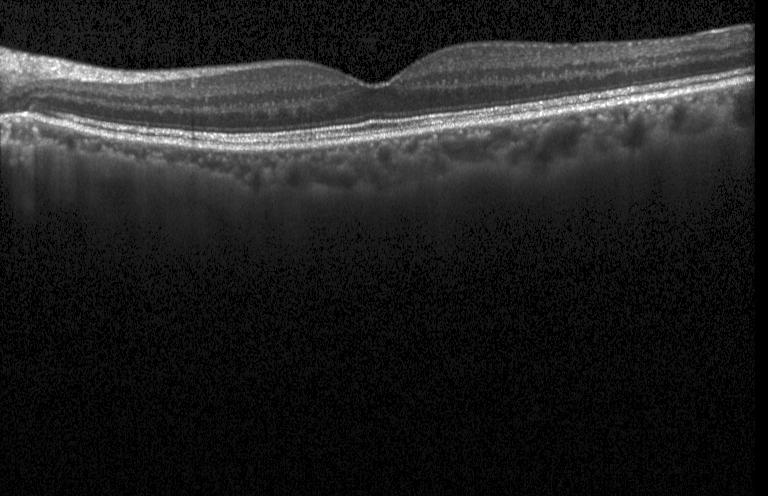
Instrument: Heidelberg Spectralis. Optical coherence tomography scan
Impression: no choroidal neovascularization, diabetic macular edema, or drusen.